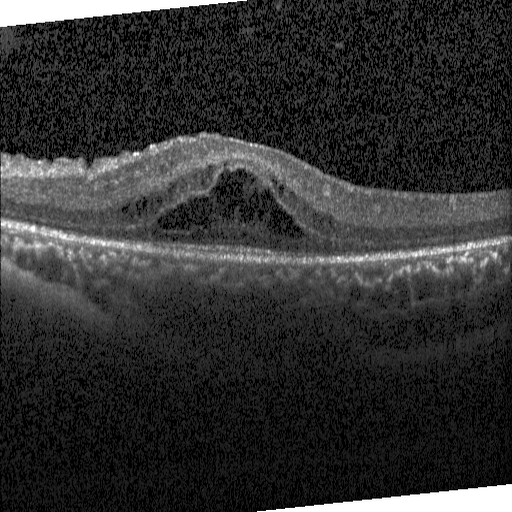

Macular scan · instrument: Heidelberg Spectralis · optical coherence tomography scan
Impression: DME.